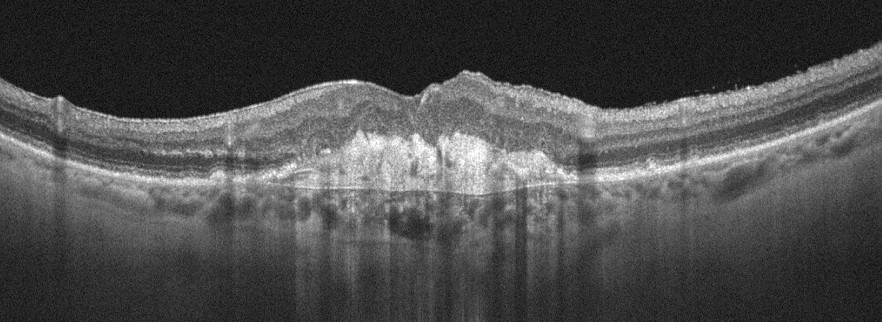 Instrument: Optovue Avanti RTVue XR; left eye; OCT B-scan; macular scan.
Macular OCT: age-related macular degeneration.